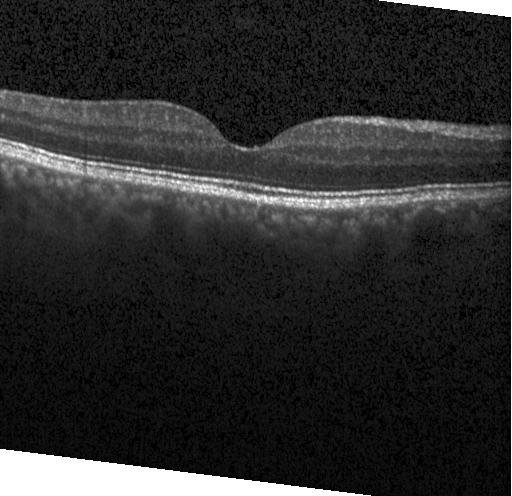
Spectral-domain optical coherence tomography, OCT B-scan, acquired on a Heidelberg Spectralis — Macular OCT: no CNV, DME, or drusen.